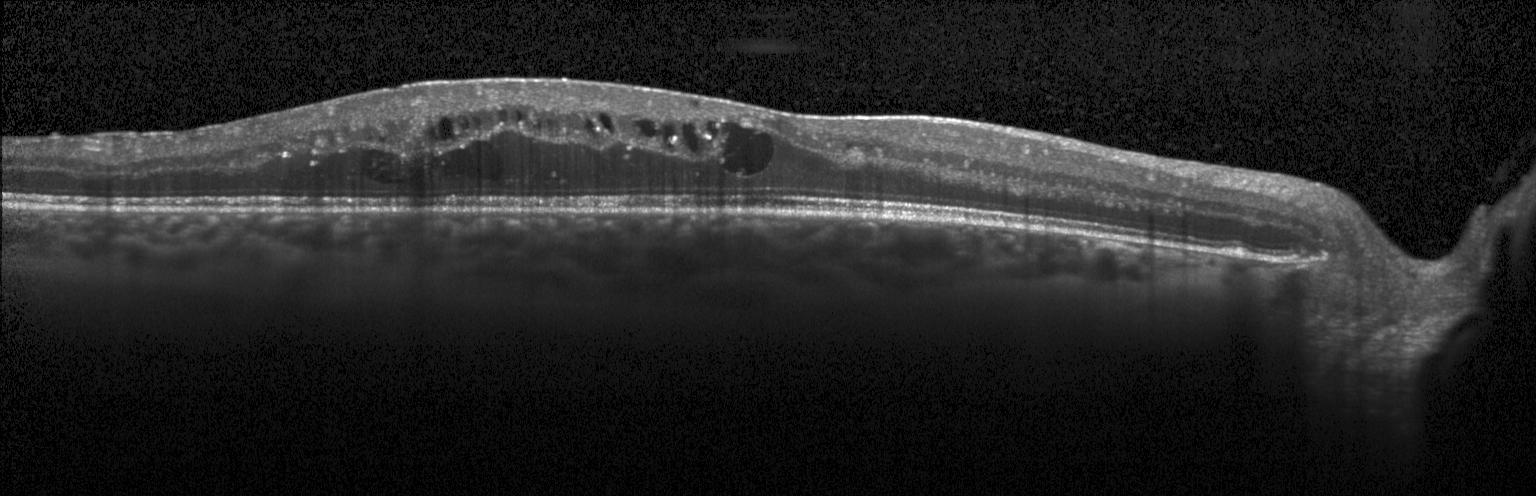

OCT B-scan · spectral-domain optical coherence tomography · horizontal scan through the fovea · instrument: Heidelberg Spectralis — Assessment: diabetic macular edema.